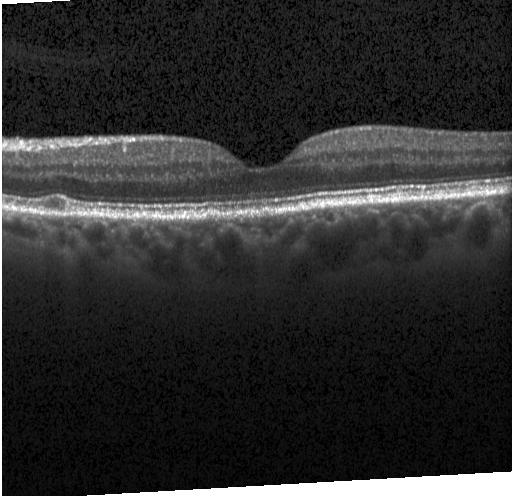

Finding: no evidence of choroidal neovascularization, diabetic macular edema, or drusen.